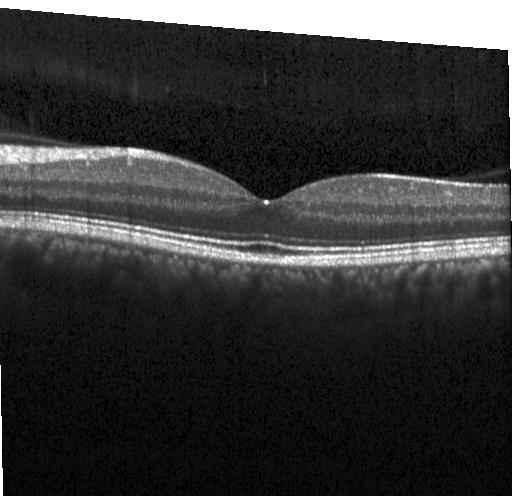

This B-scan demonstrates no choroidal neovascularization, no diabetic macular edema, and no drusen.